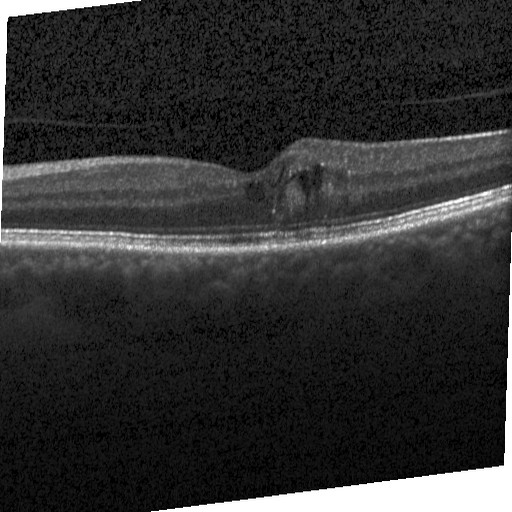
Heidelberg Spectralis OCT system · macular scan · SD-OCT · OCT B-scan. Assessment: diabetic macular edema.